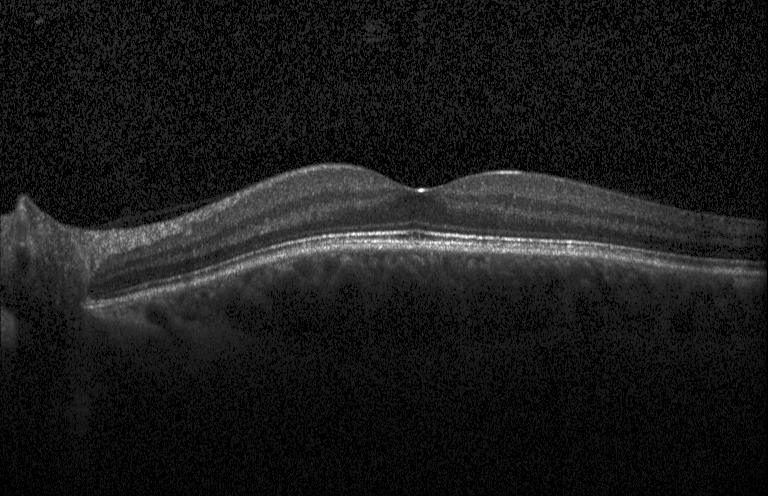 Heidelberg Spectralis; OCT line scan. The scan shows no choroidal neovascularization, diabetic macular edema, or drusen.